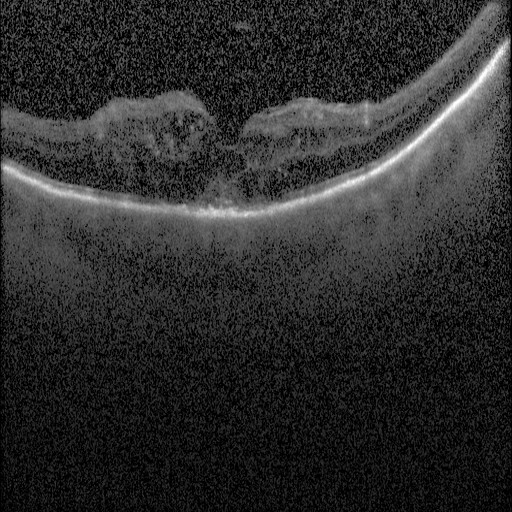 Optical coherence tomography B-scan. Heidelberg Spectralis. Centered on the fovea.
The scan shows diabetic macular edema (DME).